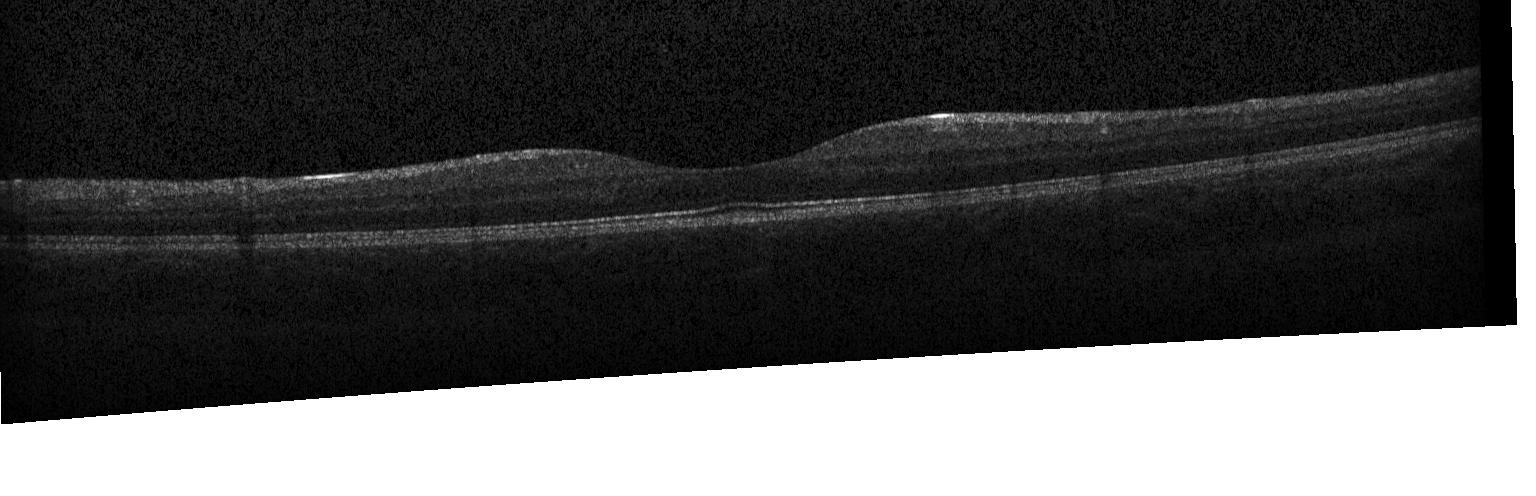
Instrument: Heidelberg Spectralis · spectral-domain optical coherence tomography · optical coherence tomography B-scan · centered on the fovea — No choroidal neovascularization, no diabetic macular edema, and no drusen.